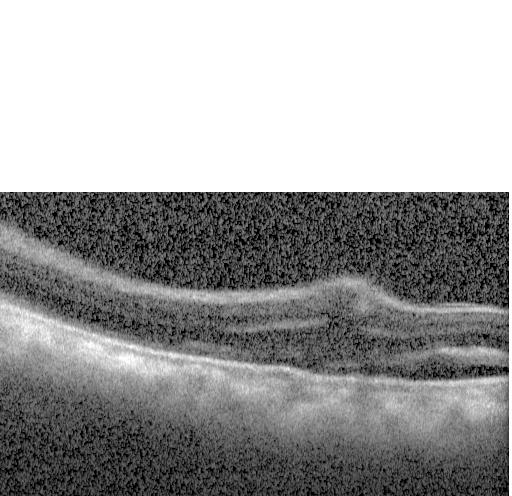

Impression: a choroidal neovascular membrane.